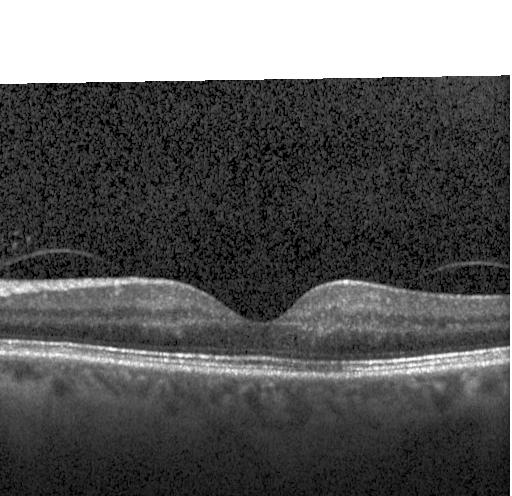

Centered on the fovea. OCT line scan. SD-OCT. Instrument: Heidelberg Spectralis — This B-scan demonstrates no choroidal neovascularization, diabetic macular edema, or drusen.